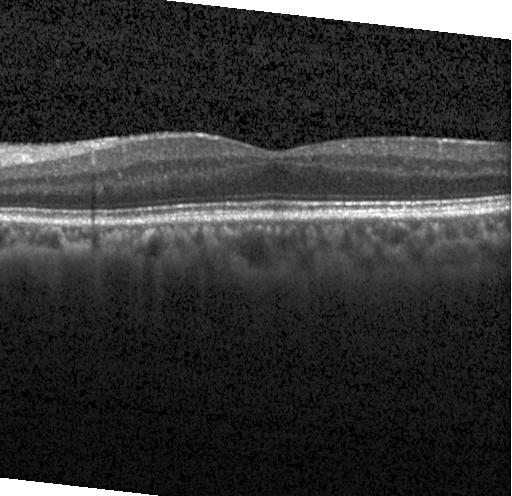 Optical coherence tomography scan. OCT finding: neither choroidal neovascularization, diabetic macular edema, nor drusen.